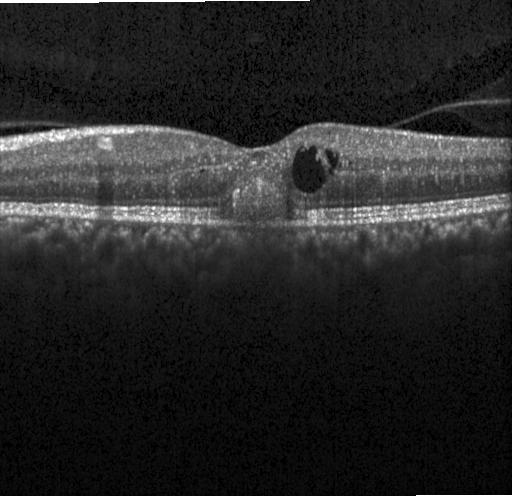 Retinal OCT B-scan; SD-OCT; horizontal scan through the fovea; Heidelberg Spectralis. Impression: a choroidal neovascular membrane.